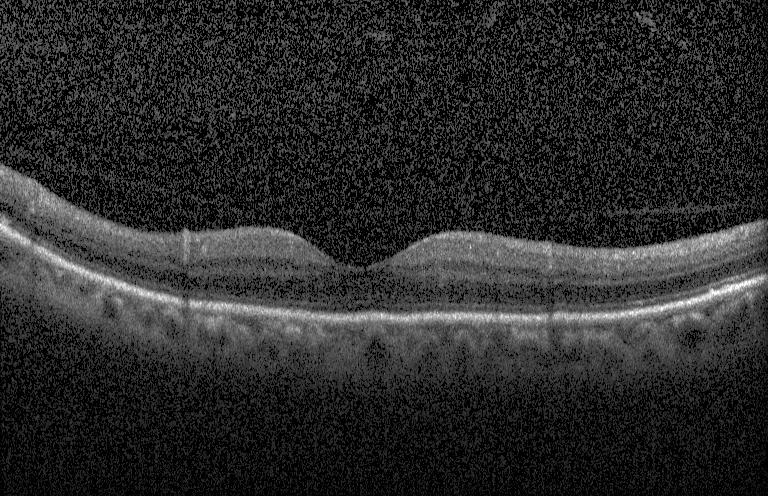
Macular scan, spectral-domain OCT, instrument: Heidelberg Spectralis, OCT line scan
OCT finding: no choroidal neovascularization, diabetic macular edema, or drusen.